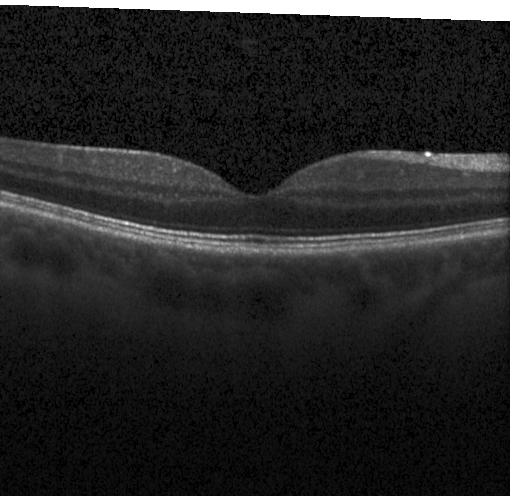

OCT finding: no CNV, no DME, and no drusen.